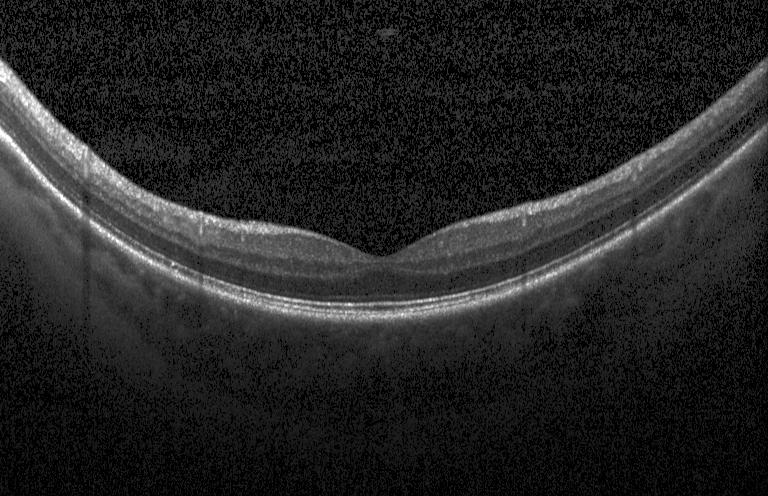

Retinal OCT B-scan. This B-scan demonstrates no choroidal neovascularization, diabetic macular edema, or drusen.